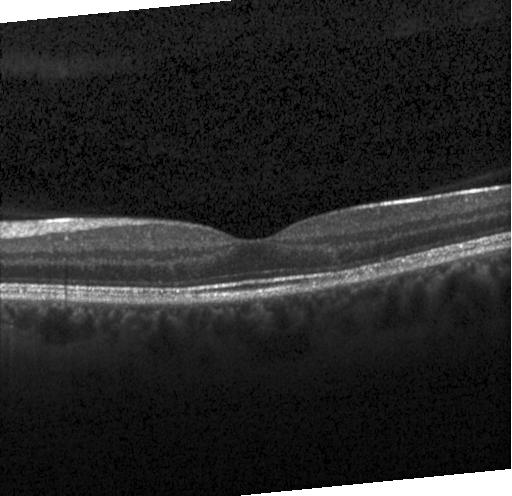 This B-scan demonstrates neither choroidal neovascularization, diabetic macular edema, nor drusen.